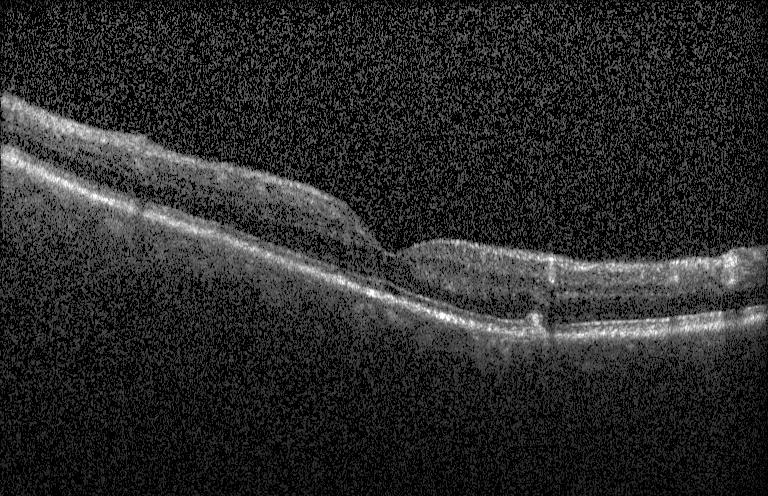
Spectral-domain optical coherence tomography. Optical coherence tomography B-scan
This B-scan demonstrates multiple drusen.